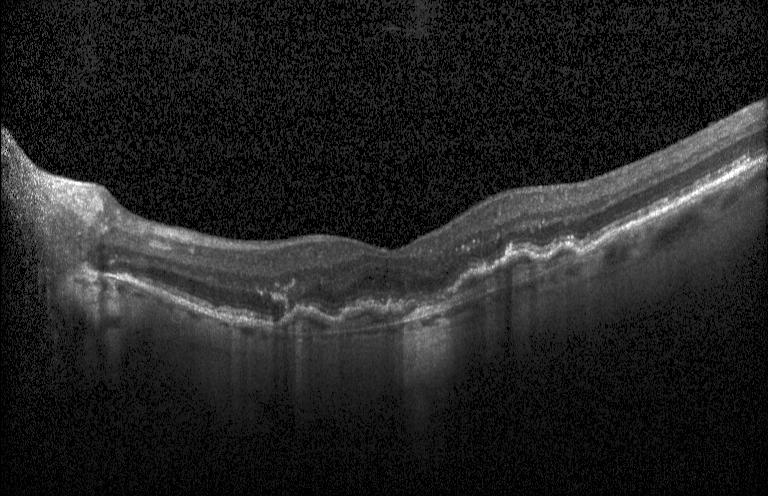

Optical coherence tomography B-scan
The scan shows choroidal neovascularization (CNV).